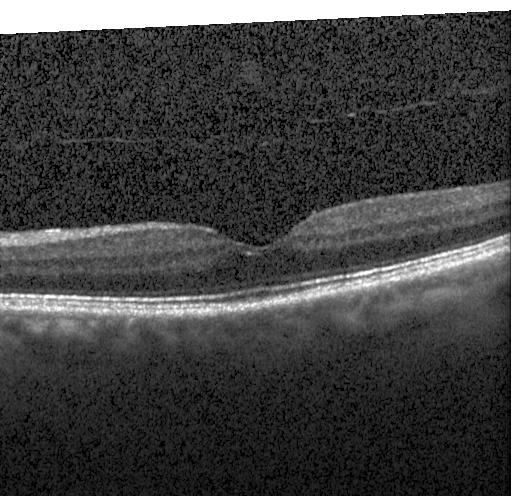 Acquired on a Heidelberg Spectralis. Optical coherence tomography scan. Horizontal scan through the fovea. Spectral-domain OCT. Neither choroidal neovascularization, diabetic macular edema, nor drusen.